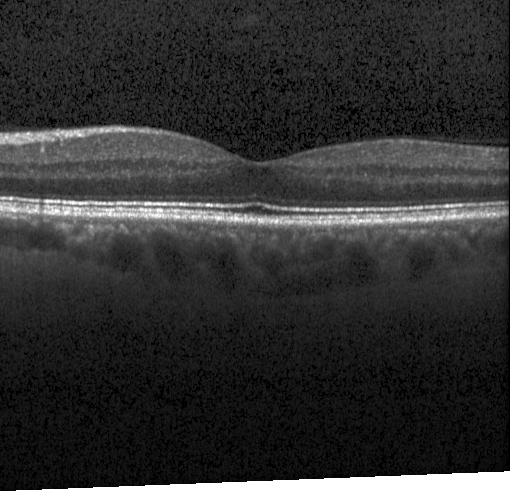

Finding: no evidence of choroidal neovascularization, diabetic macular edema, or drusen.